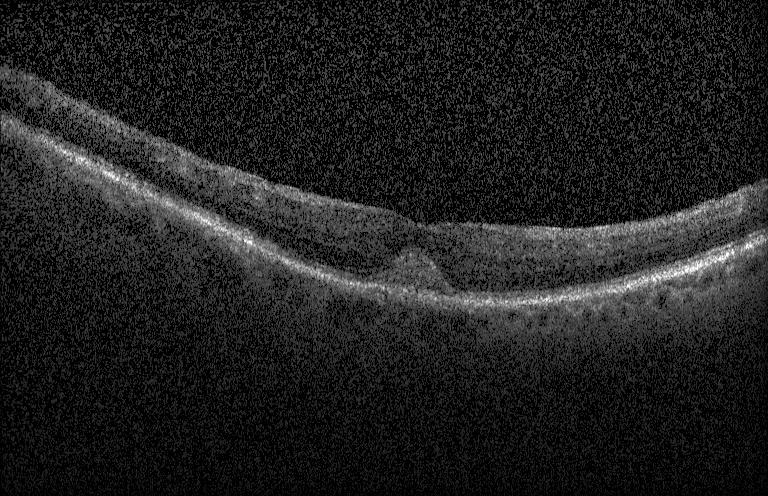
Retinal OCT cross-section; spectral-domain OCT. Finding: choroidal neovascularization.